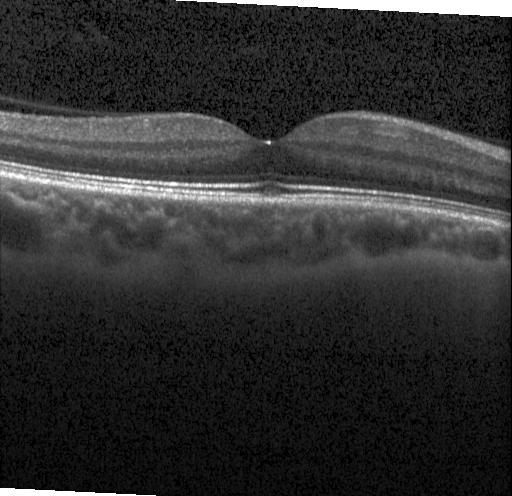
Retinal OCT cross-section showing no evidence of CNV, DME, or drusen.